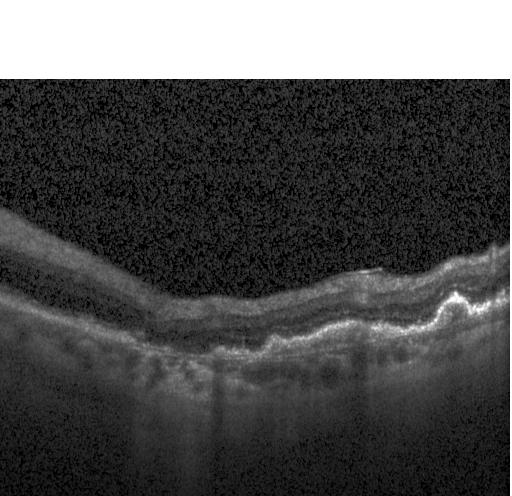
Diagnosis: choroidal neovascularization.